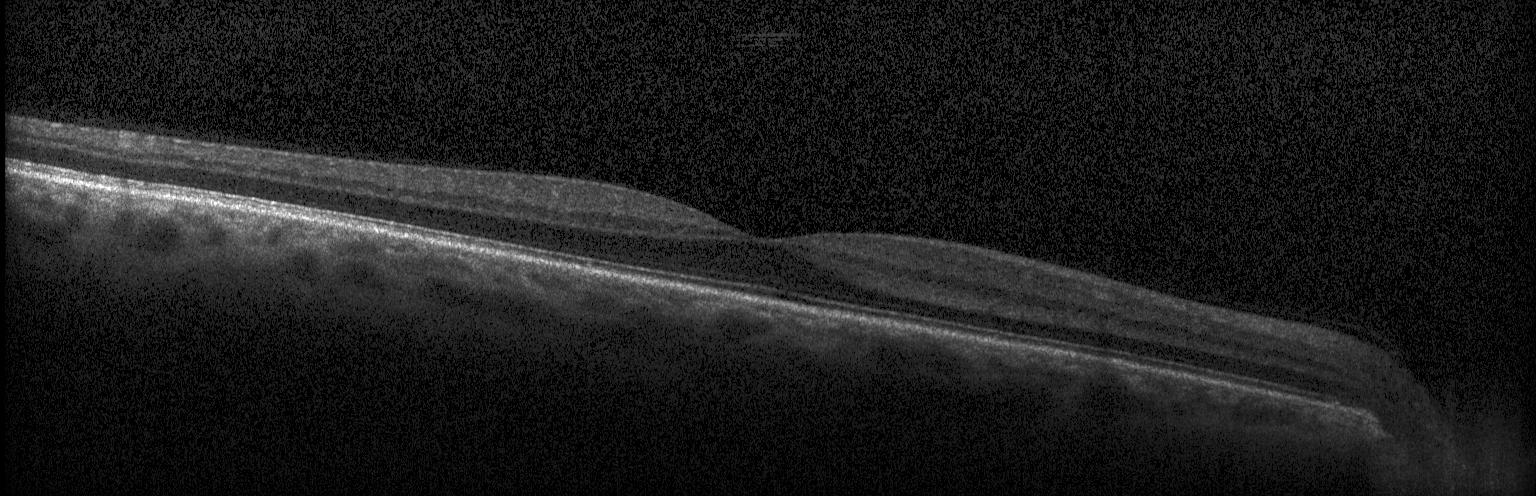 Heidelberg Spectralis. Macular scan. Optical coherence tomography B-scan. Spectral-domain optical coherence tomography — Dx: no evidence of choroidal neovascularization, diabetic macular edema, or drusen.